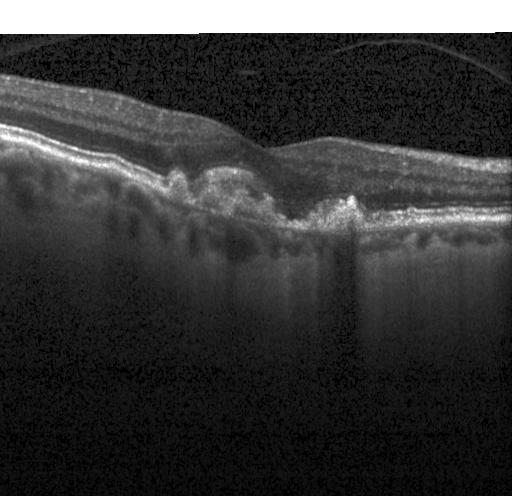

This B-scan demonstrates a choroidal neovascular membrane.